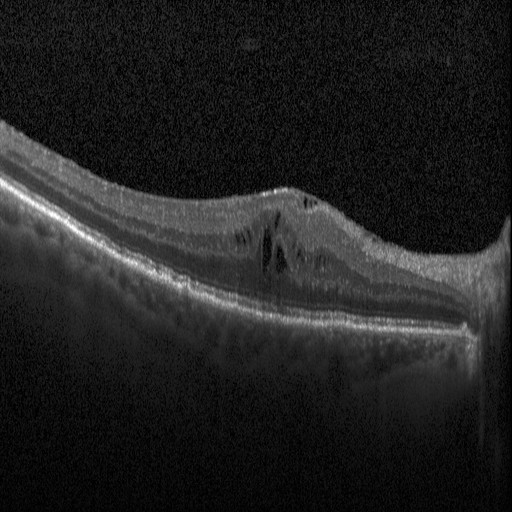 Heidelberg Spectralis OCT system, optical coherence tomography B-scan. Diabetic macular edema.